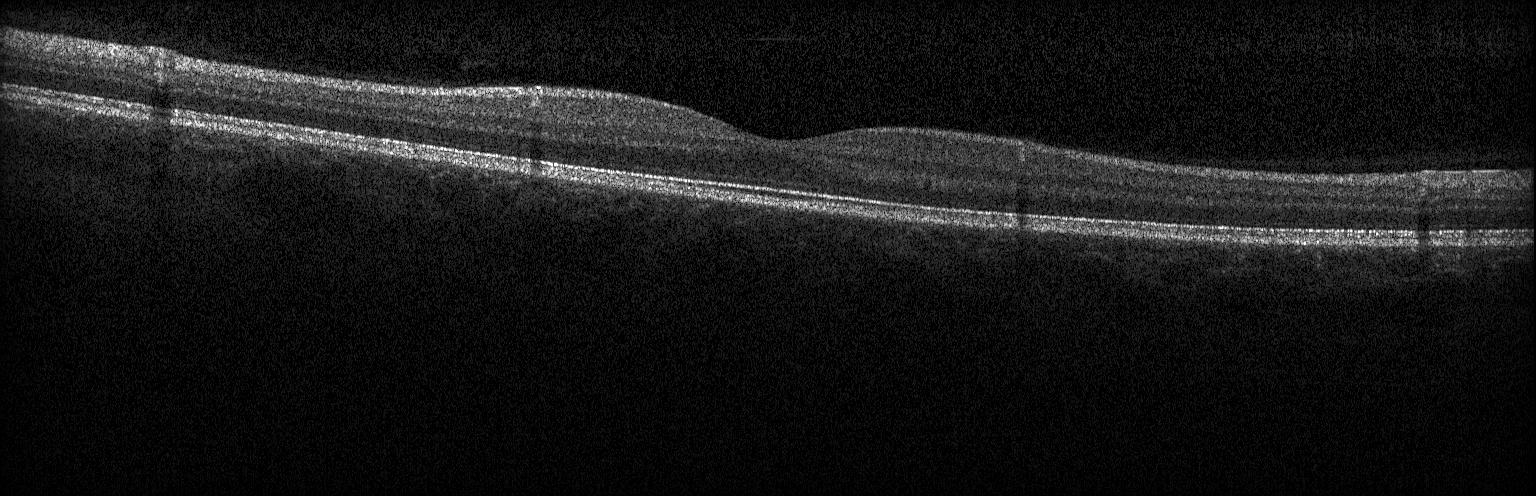 Optical coherence tomography scan
No choroidal neovascularization, diabetic macular edema, or drusen.